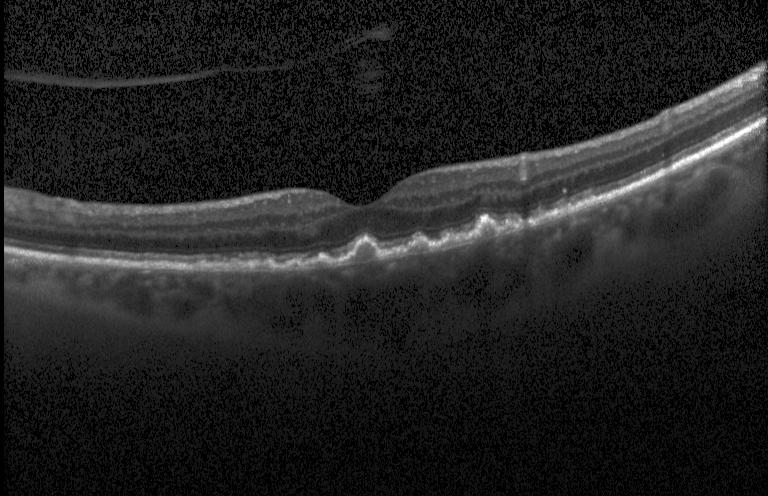

Spectral-domain OCT · retinal OCT B-scan · fovea-centered · Heidelberg Spectralis OCT system — Assessment: multiple drusen.